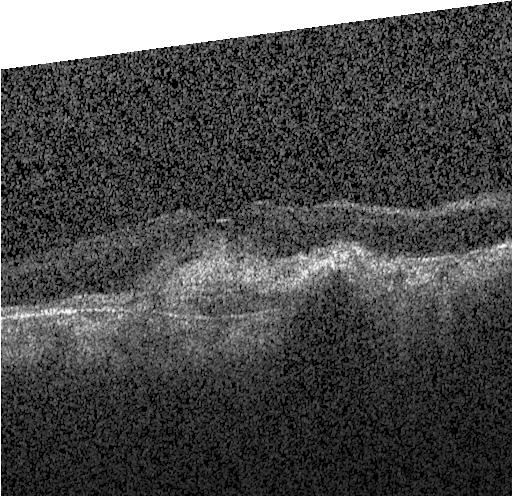
Centered on the fovea · spectral-domain OCT · retinal OCT B-scan.
This B-scan demonstrates choroidal neovascularization (CNV).